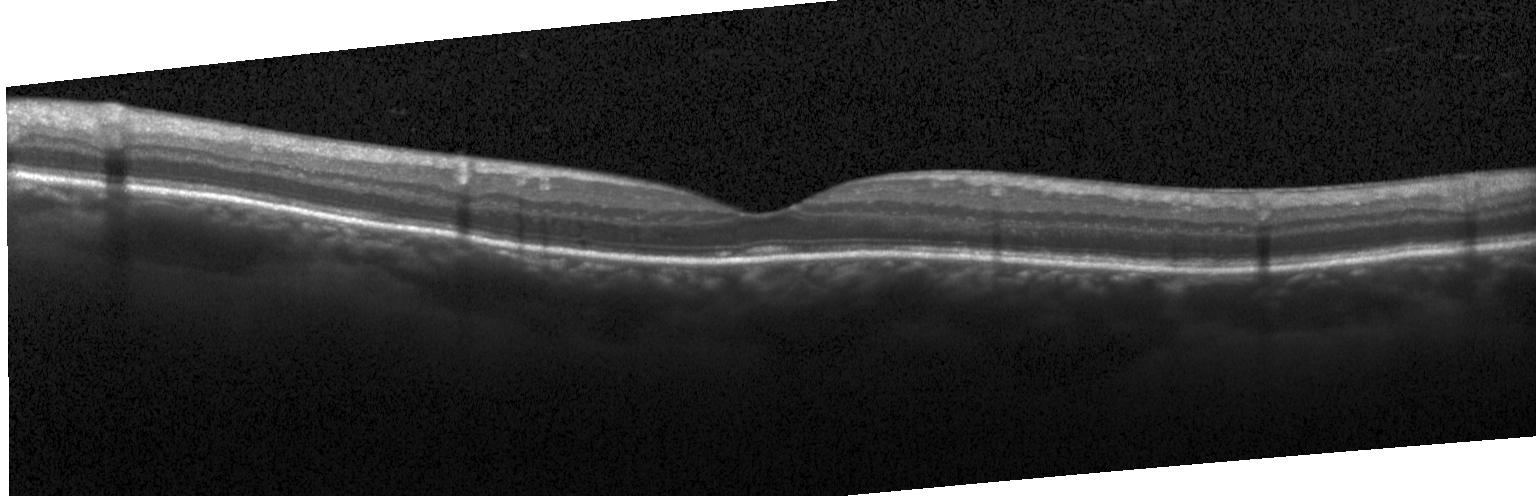

Dx: no choroidal neovascularization, no diabetic macular edema, and no drusen.